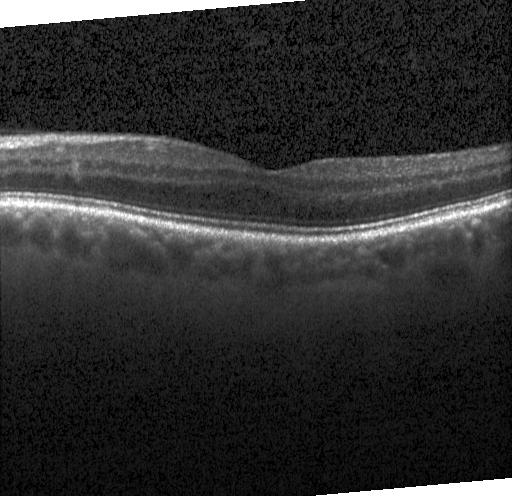 Retinal OCT cross-section
This B-scan demonstrates no evidence of CNV, DME, or drusen.